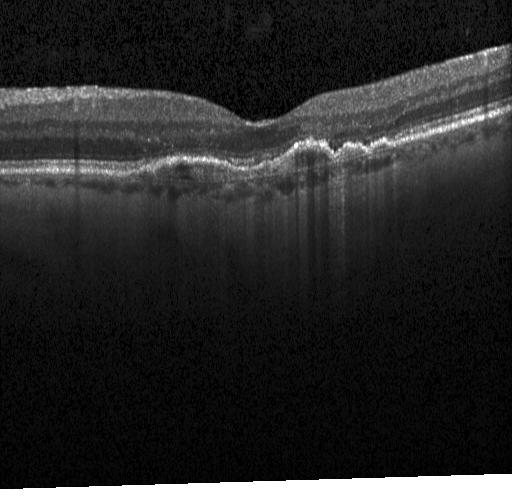
Optical coherence tomography scan · through the macula · spectral-domain OCT — Impression: choroidal neovascularization (CNV).